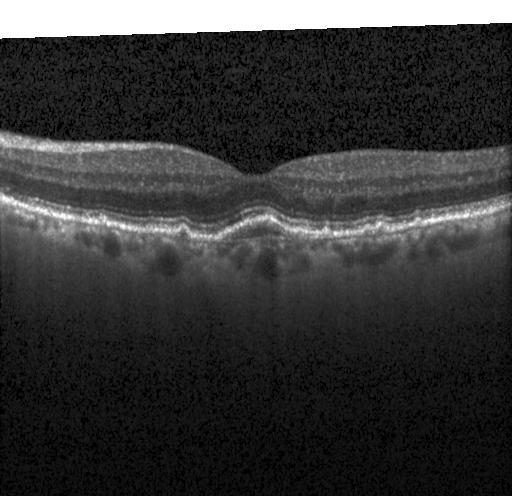 Macular scan · spectral-domain optical coherence tomography · optical coherence tomography B-scan · instrument: Heidelberg Spectralis.
Assessment: a choroidal neovascular membrane.